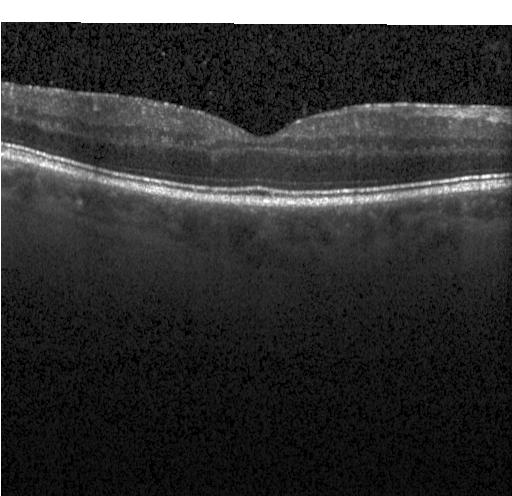
Horizontal scan through the fovea, retinal OCT cross-section, instrument: Heidelberg Spectralis, spectral-domain OCT.
Impression: no evidence of CNV, DME, or drusen.